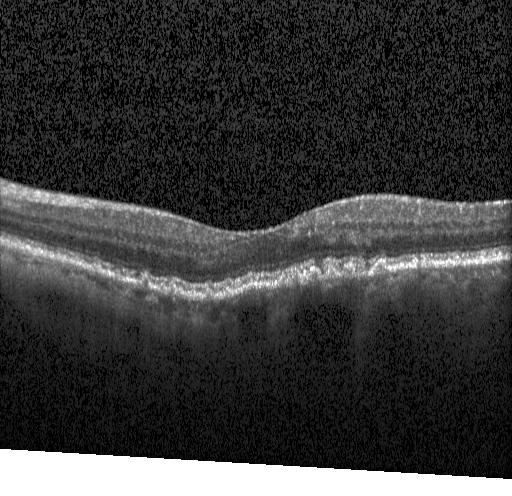
OCT B-scan; Heidelberg Spectralis; spectral-domain OCT — Finding: drusen.